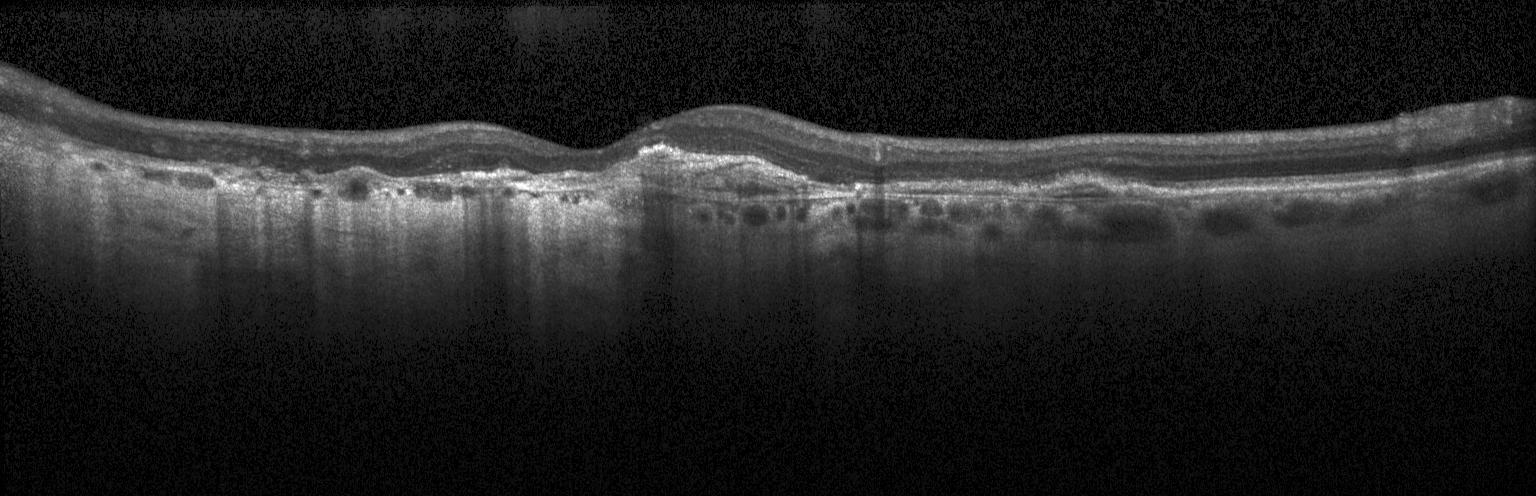

Instrument: Heidelberg Spectralis, optical coherence tomography scan, through the macula. This B-scan demonstrates a choroidal neovascular membrane.